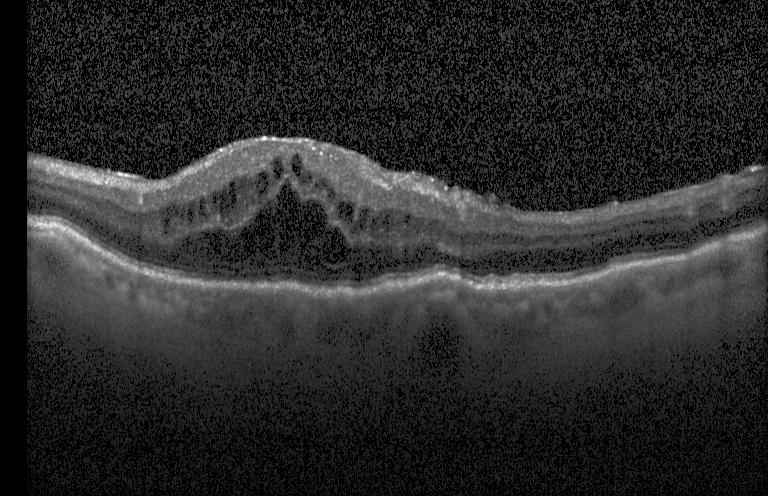
Optical coherence tomography B-scan. Finding: diabetic macular edema.